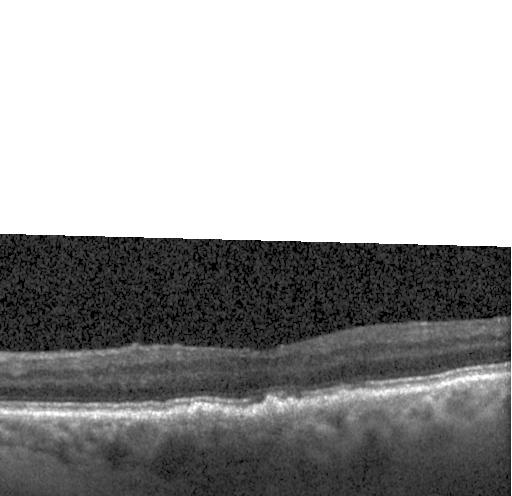
Retinal OCT B-scan. Spectral-domain OCT. Horizontal scan through the fovea. Instrument: Heidelberg Spectralis.
This B-scan demonstrates multiple drusen.